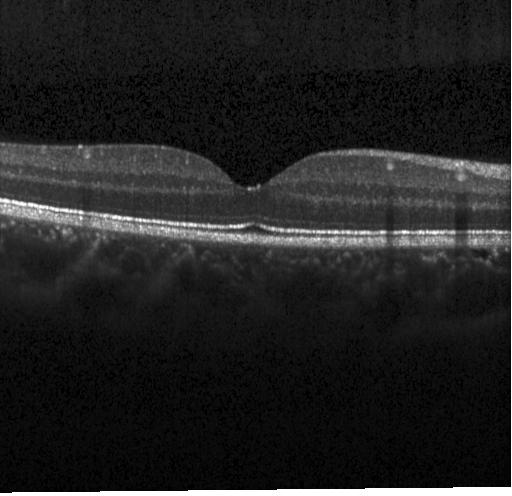
Optical coherence tomography B-scan; spectral-domain OCT; through the macula; Heidelberg Spectralis OCT system. The scan shows no CNV, DME, or drusen.